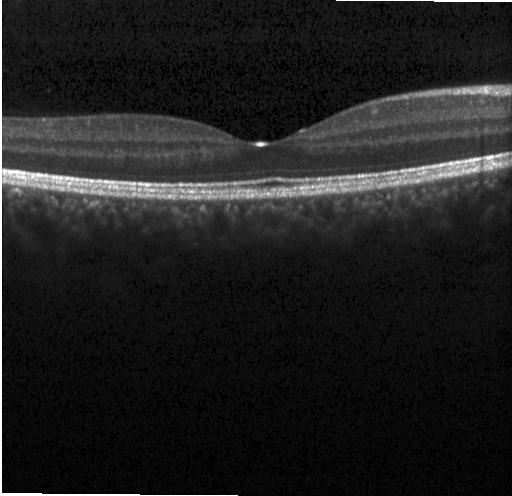
Impression: neither choroidal neovascularization, diabetic macular edema, nor drusen.